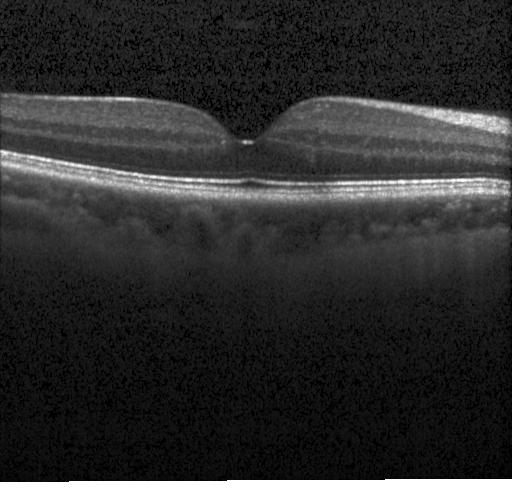
Horizontal scan through the fovea · retinal OCT B-scan · acquired on a Heidelberg Spectralis · spectral-domain OCT. Diagnosis: no choroidal neovascularization, no diabetic macular edema, and no drusen.